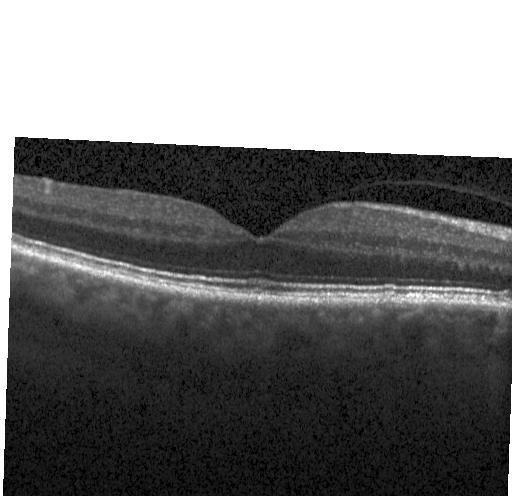 No CNV, no DME, and no drusen.